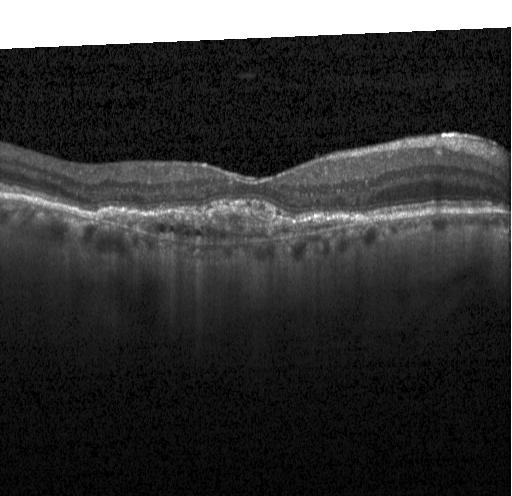

Horizontal scan through the fovea, OCT B-scan — Finding: choroidal neovascularization (CNV).